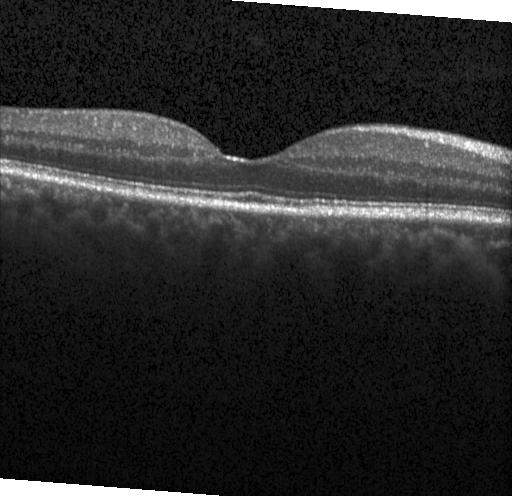

Diagnosis: no choroidal neovascularization, no diabetic macular edema, and no drusen.